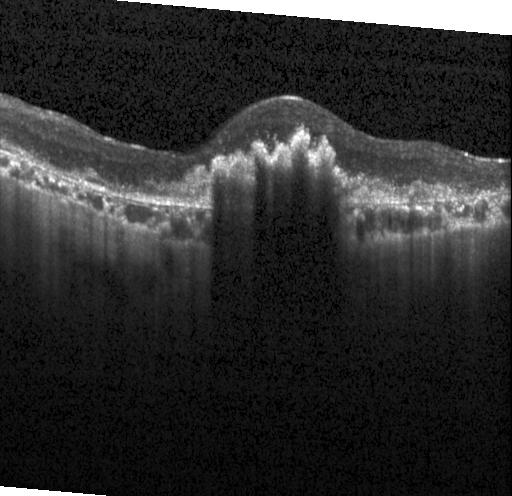

OCT B-scan showing CNV.